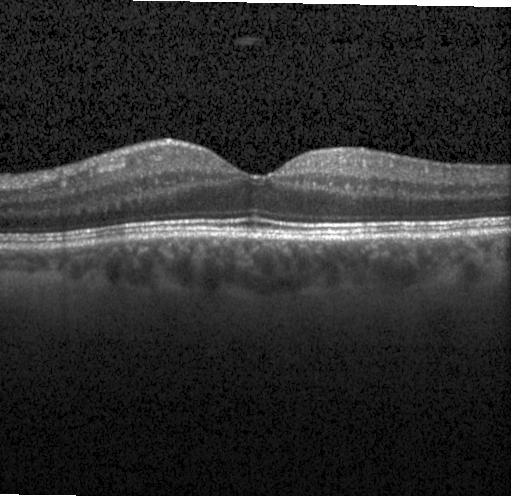

Retinal OCT B-scan · fovea-centered. Diagnosis: neither CNV, DME, nor drusen.